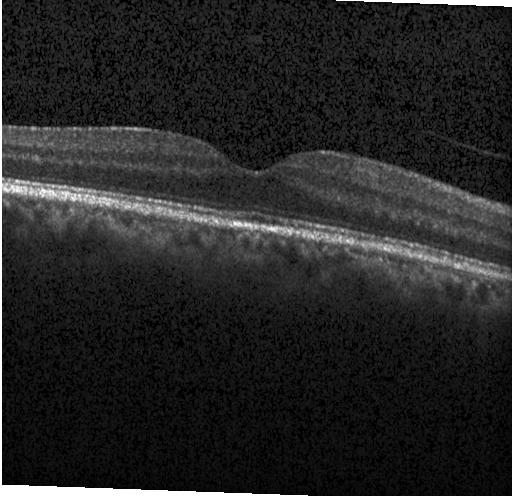
Retinal OCT B-scan, Heidelberg Spectralis
Dx: no CNV, DME, or drusen.